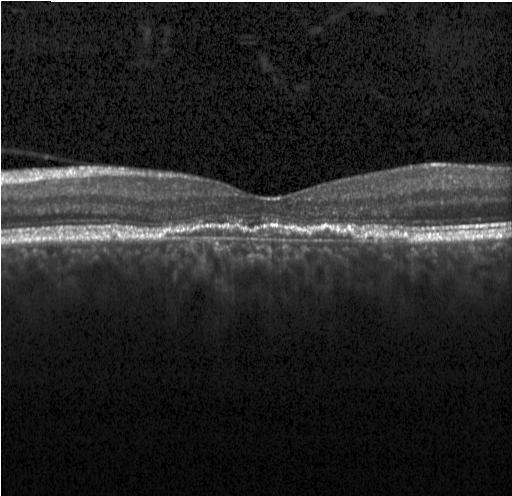
Retinal OCT cross-section. Horizontal scan through the fovea. SD-OCT.
OCT finding: a choroidal neovascular membrane.